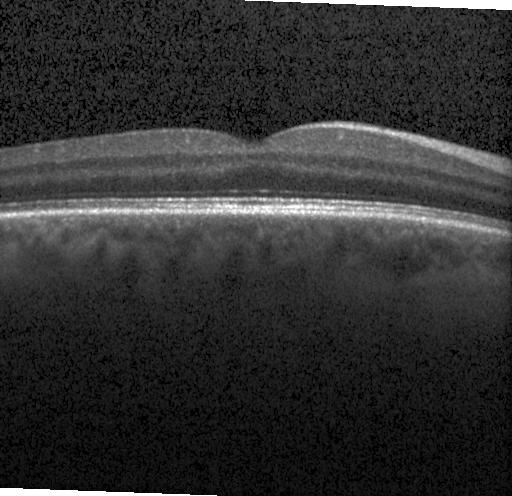 Macular scan; instrument: Heidelberg Spectralis; retinal OCT cross-section
No evidence of choroidal neovascularization, diabetic macular edema, or drusen.